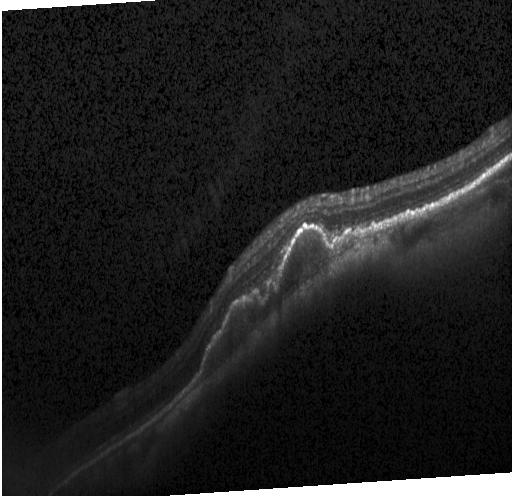

Finding: a choroidal neovascular membrane.